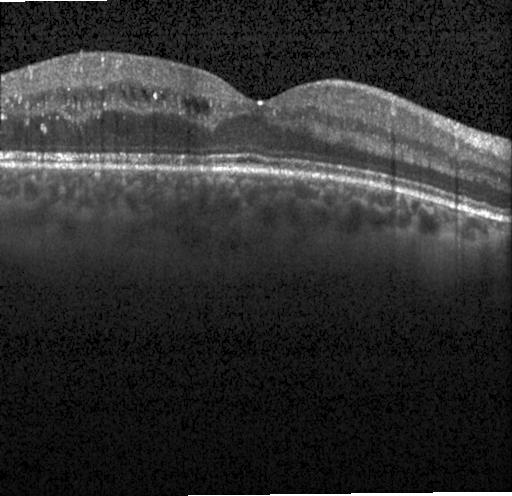 Fovea-centered · spectral-domain optical coherence tomography · OCT B-scan · acquired on a Heidelberg Spectralis
OCT finding: diabetic macular edema.